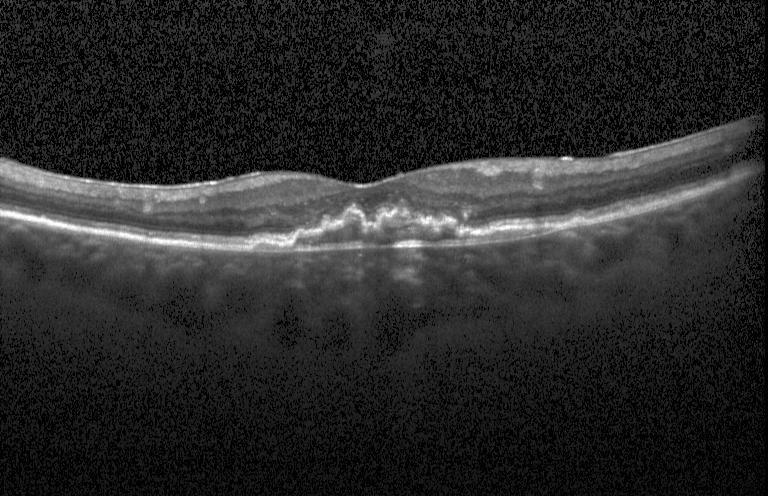 Retinal OCT cross-section showing CNV.